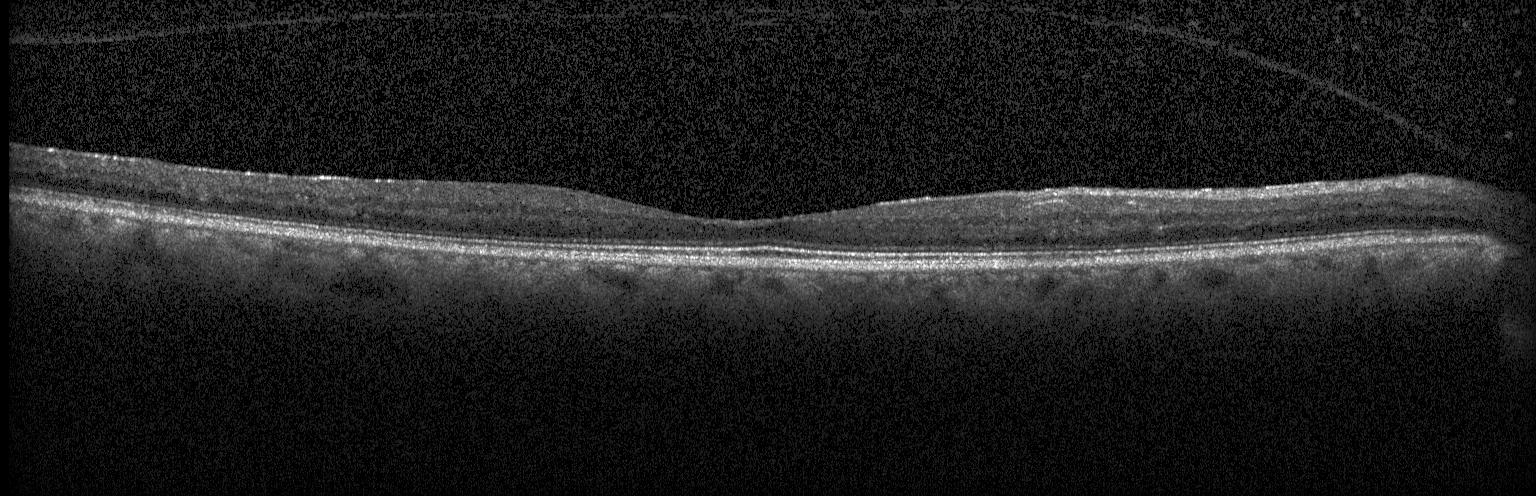

Dx: no choroidal neovascularization, no diabetic macular edema, and no drusen.